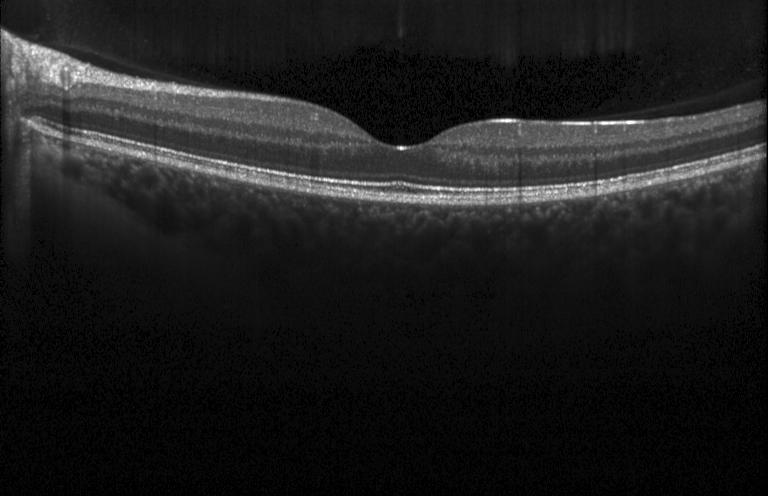

Instrument: Heidelberg Spectralis · spectral-domain optical coherence tomography · optical coherence tomography B-scan.
Finding: no choroidal neovascularization, no diabetic macular edema, and no drusen.